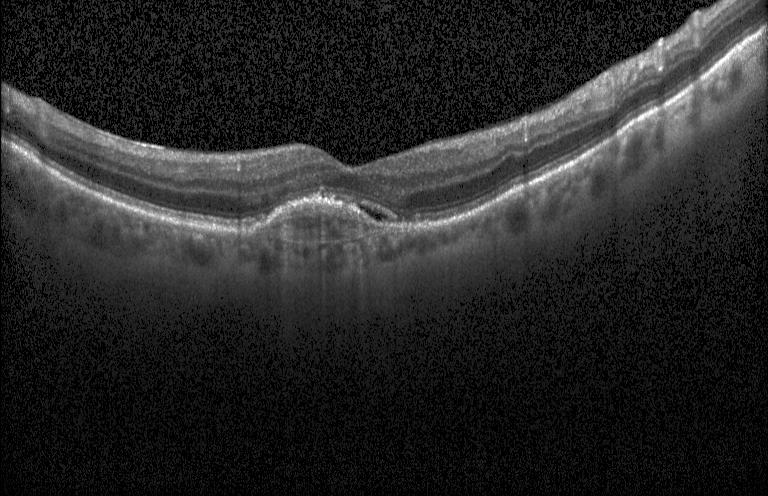 Diagnosis: choroidal neovascularization (CNV).